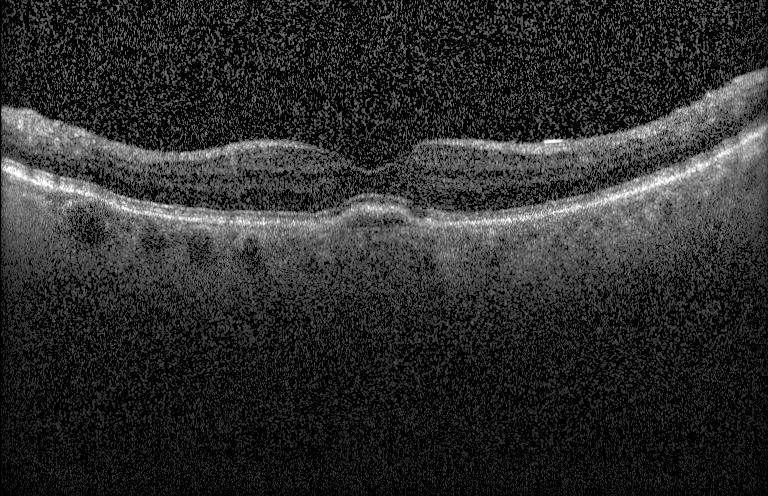
Spectral-domain OCT; macular scan; retinal OCT cross-section
Diagnosis: choroidal neovascularization (CNV).